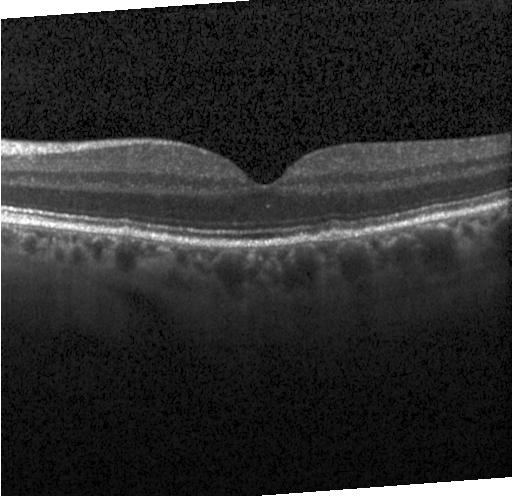
The scan shows drusen.